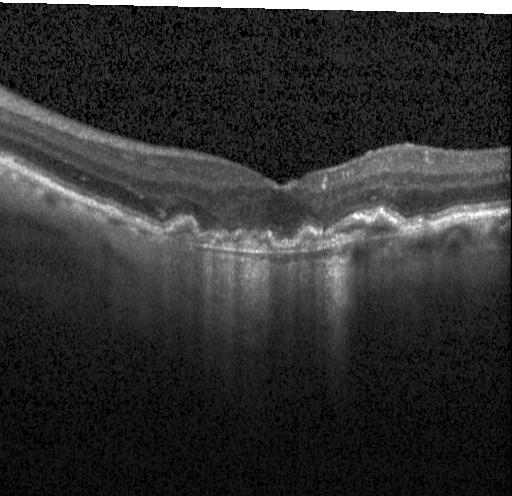

Spectral-domain optical coherence tomography. Macular scan. Instrument: Heidelberg Spectralis. Optical coherence tomography scan
Dx: a choroidal neovascular membrane.